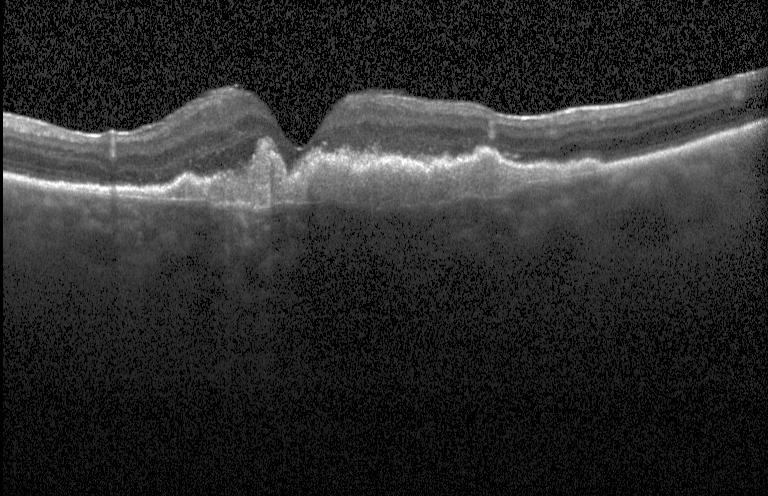

OCT line scan, SD-OCT — Dx: a choroidal neovascular membrane.